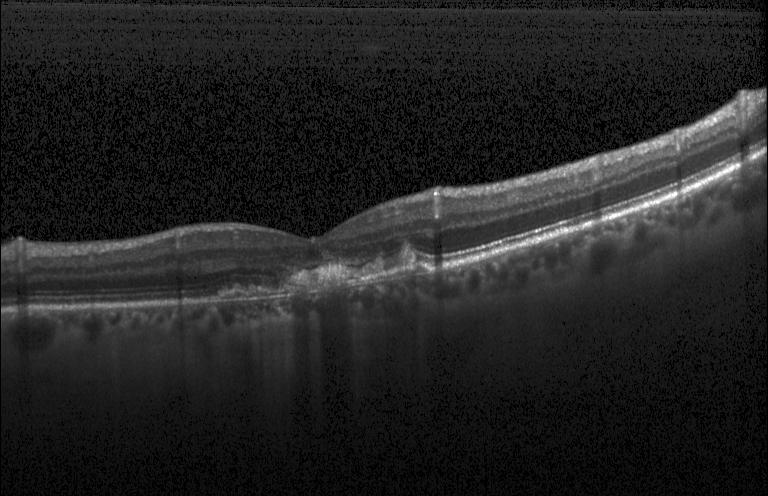

Retinal OCT cross-section · through the macula. Diagnosis: choroidal neovascularization.